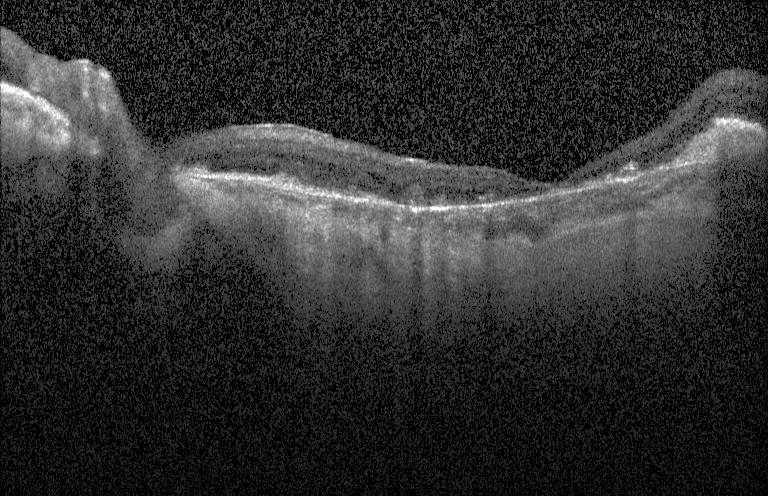 Horizontal scan through the fovea, Heidelberg Spectralis OCT system, optical coherence tomography scan
Finding: CNV.